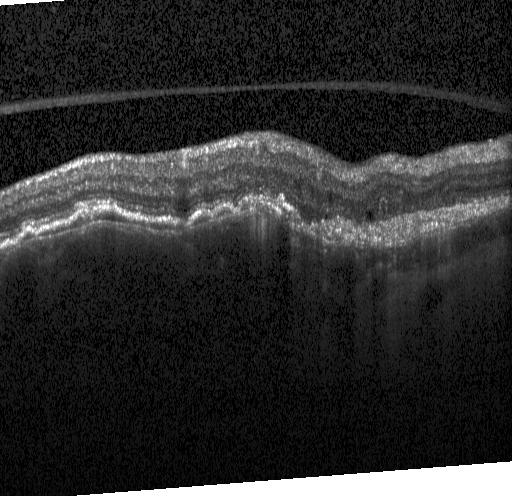

OCT B-scan, through the macula.
Choroidal neovascularization.